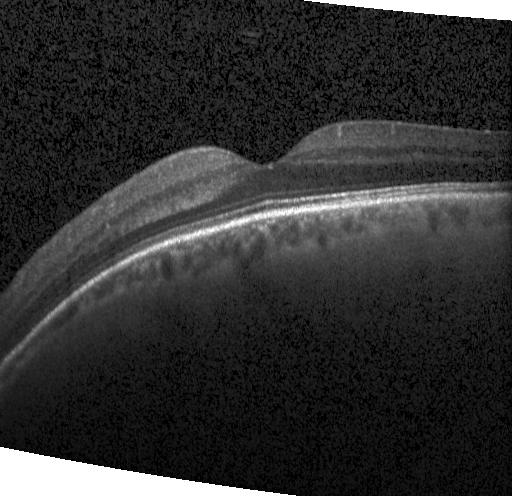 No CNV, no DME, and no drusen.